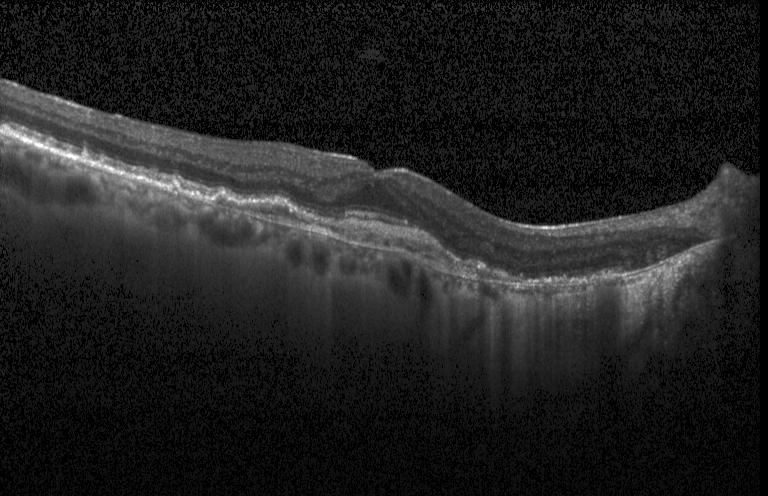

OCT B-scan, fovea-centered.
Macular OCT: a choroidal neovascular membrane.